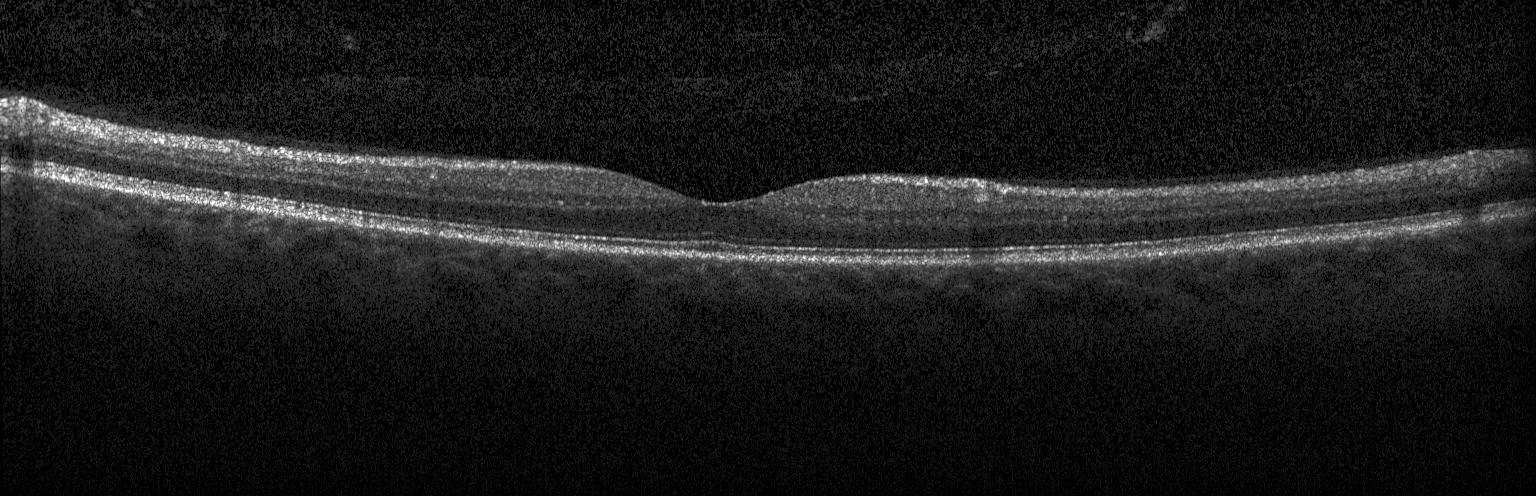

Finding: no CNV, DME, or drusen.